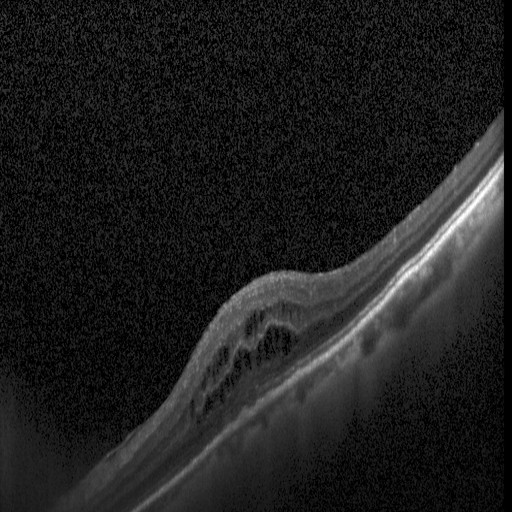
OCT line scan; spectral-domain optical coherence tomography; horizontal scan through the fovea — Diabetic macular edema.